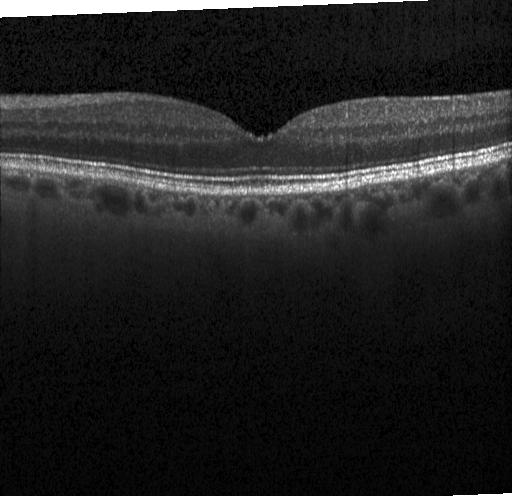

Optical coherence tomography scan · spectral-domain OCT. Dx: no evidence of choroidal neovascularization, diabetic macular edema, or drusen.